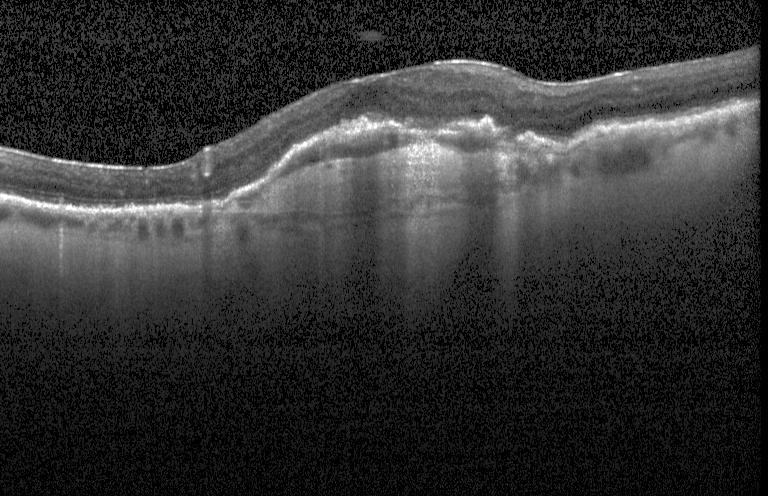
Macular OCT demonstrating CNV.